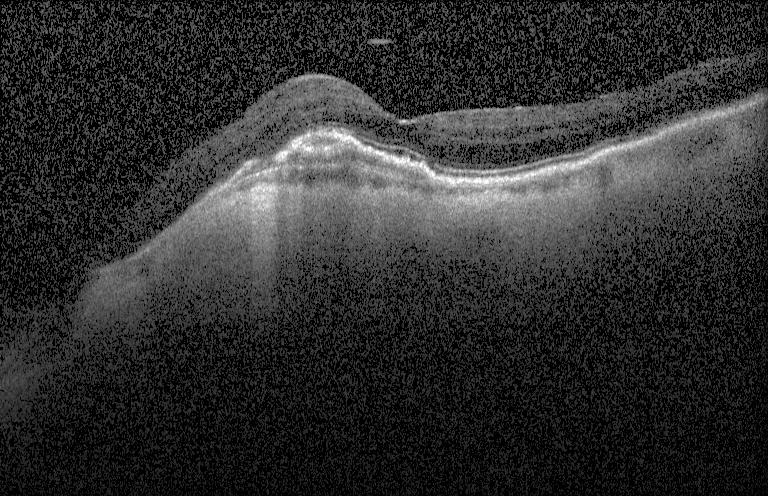 Diagnosis: a choroidal neovascular membrane.